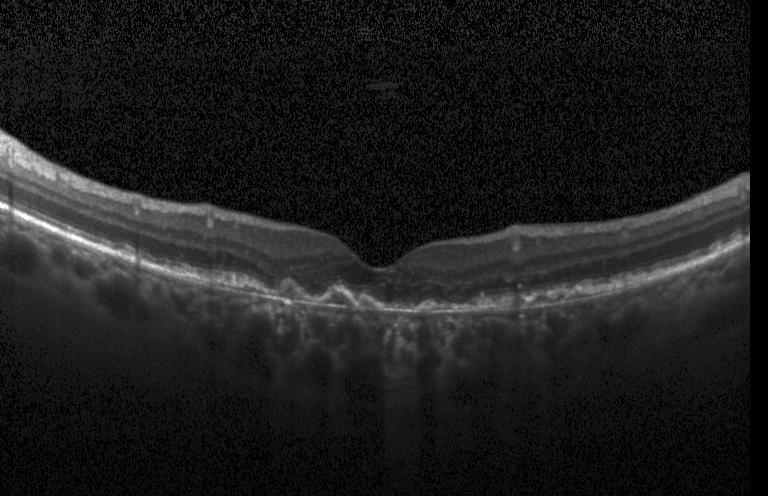

This B-scan demonstrates a choroidal neovascular membrane.